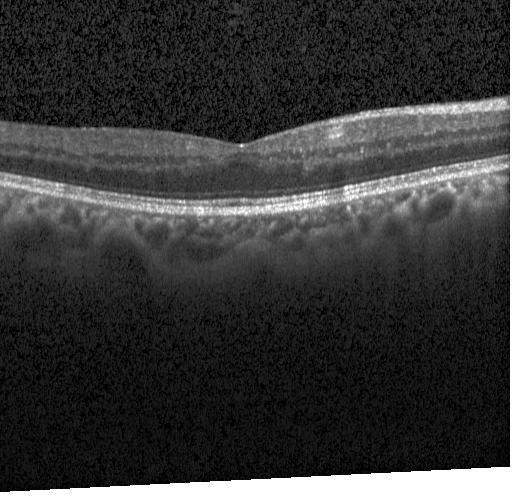
Diagnosis: neither choroidal neovascularization, diabetic macular edema, nor drusen.